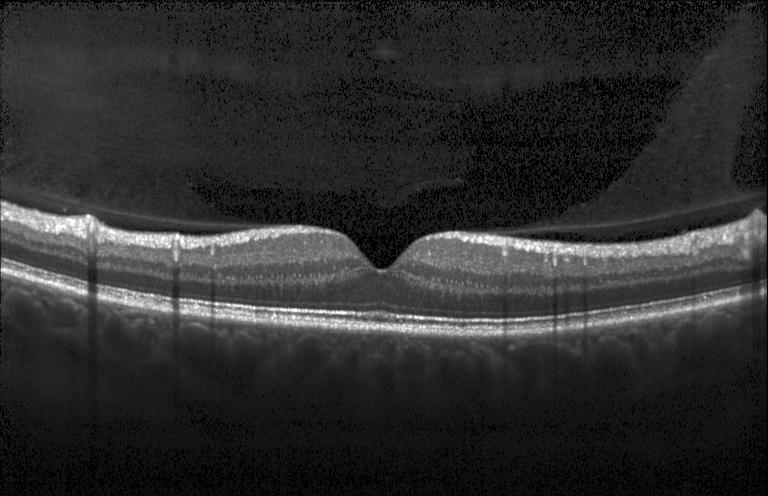

Optical coherence tomography B-scan; through the macula; acquired on a Heidelberg Spectralis
The scan shows no choroidal neovascularization, diabetic macular edema, or drusen.